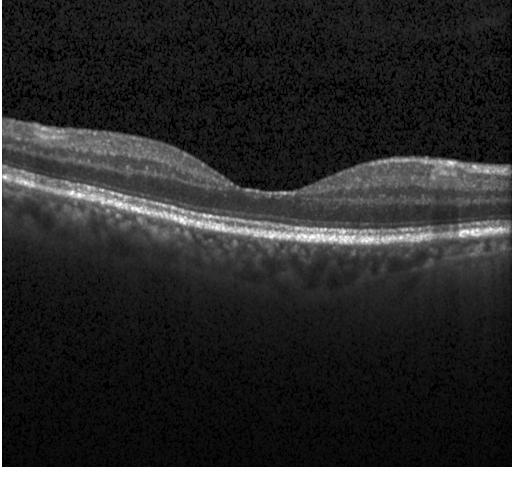

Optical coherence tomography B-scan; macular scan — Impression: no CNV, no DME, and no drusen.